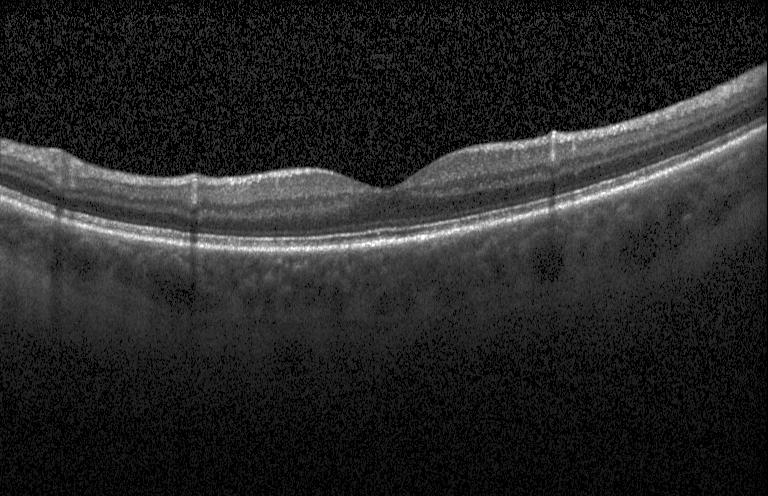

Instrument: Heidelberg Spectralis, OCT B-scan.
Finding: neither choroidal neovascularization, diabetic macular edema, nor drusen.